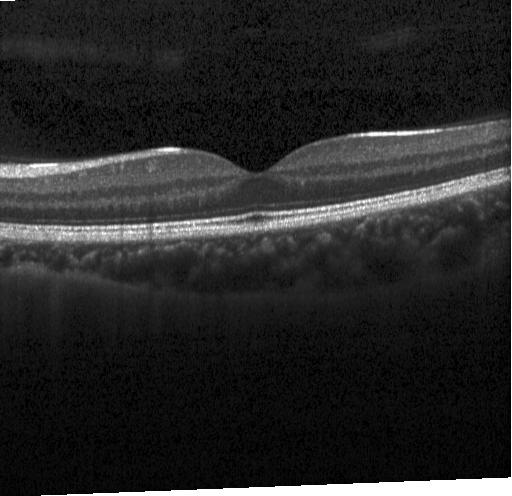
No evidence of choroidal neovascularization, diabetic macular edema, or drusen.